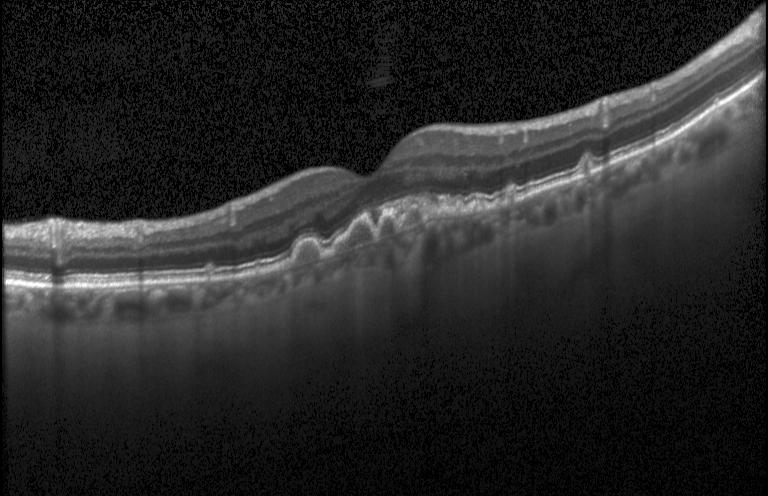 Multiple drusen.